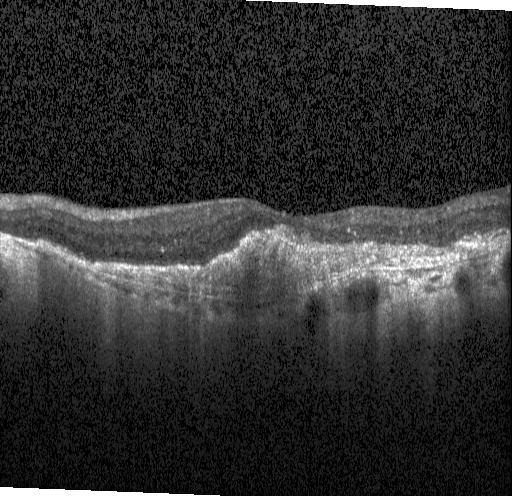 Acquired on a Heidelberg Spectralis · retinal OCT B-scan · SD-OCT
This B-scan demonstrates CNV.